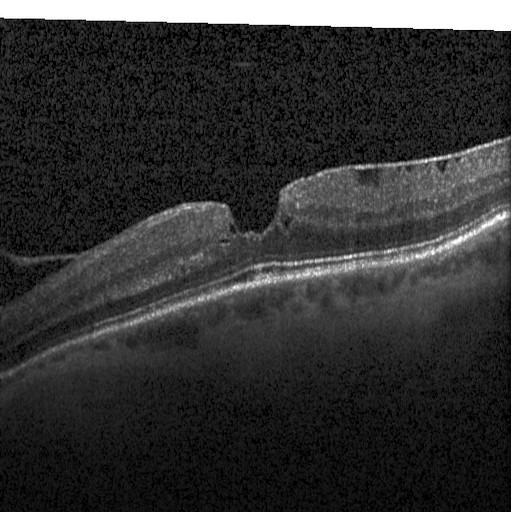
DME.